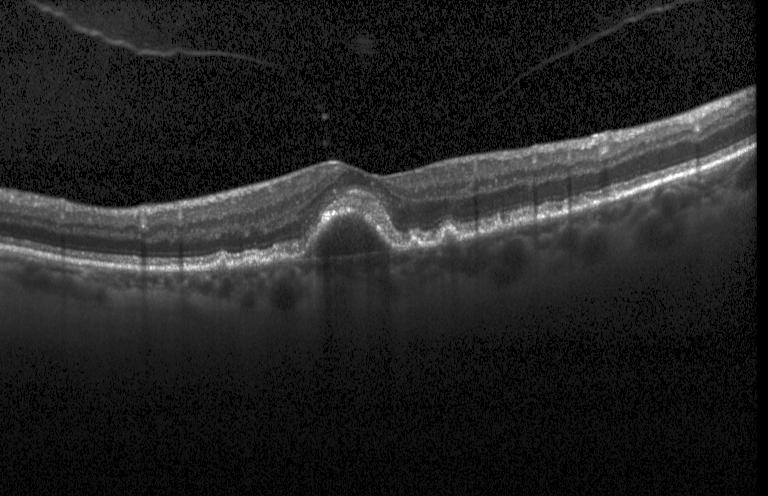 Optical coherence tomography B-scan — Finding: a choroidal neovascular membrane.